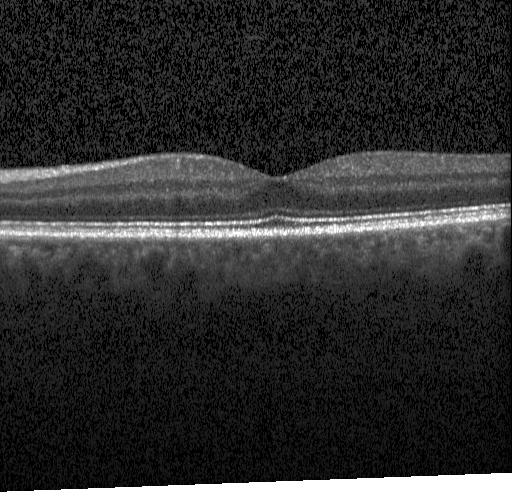
OCT scan showing no CNV, DME, or drusen.